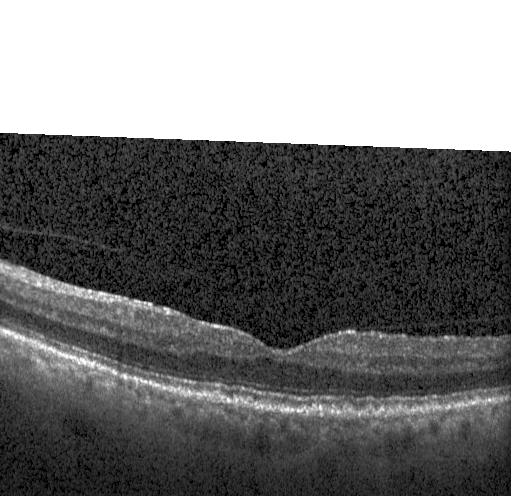 Instrument: Heidelberg Spectralis. SD-OCT. Optical coherence tomography scan.
The scan shows multiple drusen.